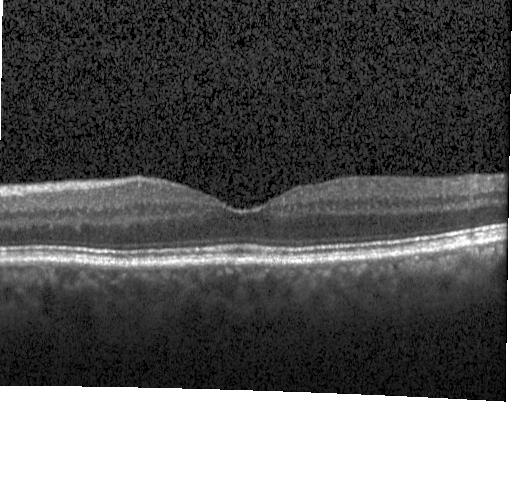

Diagnosis: no choroidal neovascularization, diabetic macular edema, or drusen.